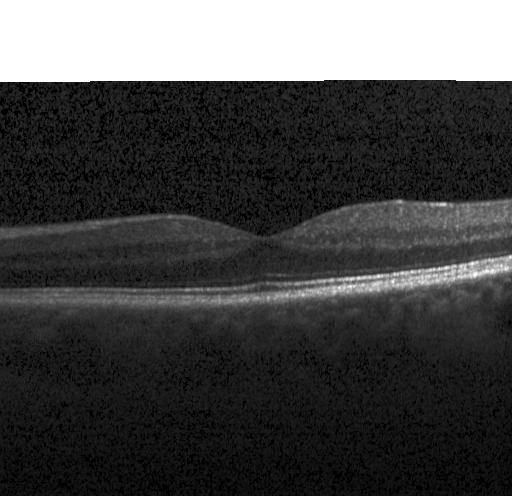 Retinal OCT B-scan. OCT finding: no choroidal neovascularization, diabetic macular edema, or drusen.